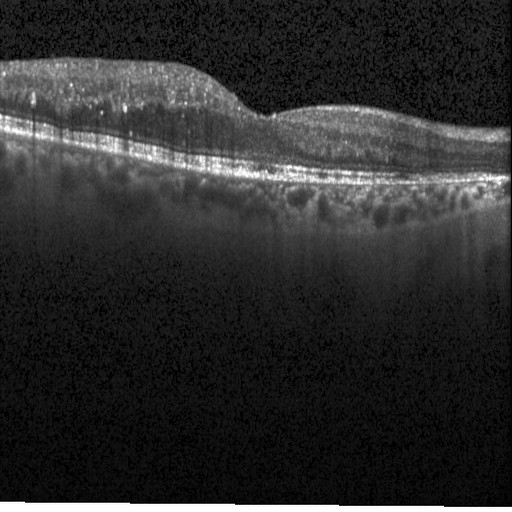

Finding: diabetic macular edema.